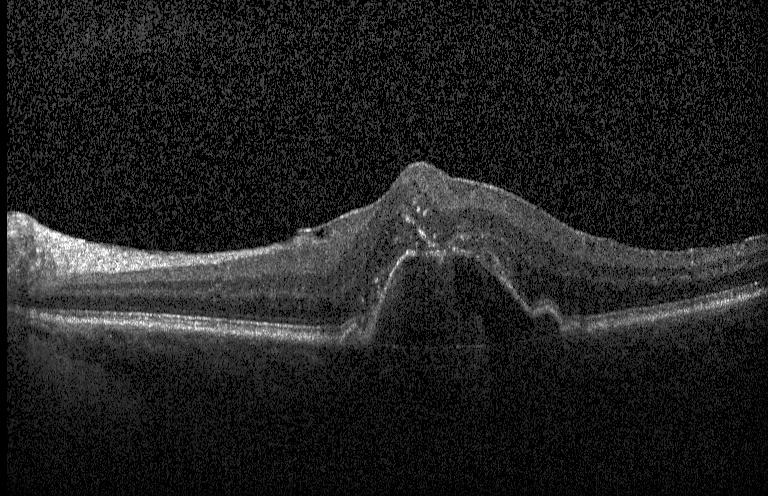 Retinal OCT cross-section. Macular scan. SD-OCT. Finding: a choroidal neovascular membrane.